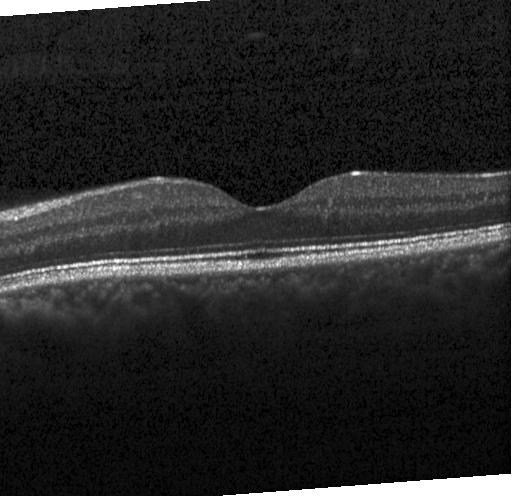

Impression: no choroidal neovascularization, no diabetic macular edema, and no drusen.